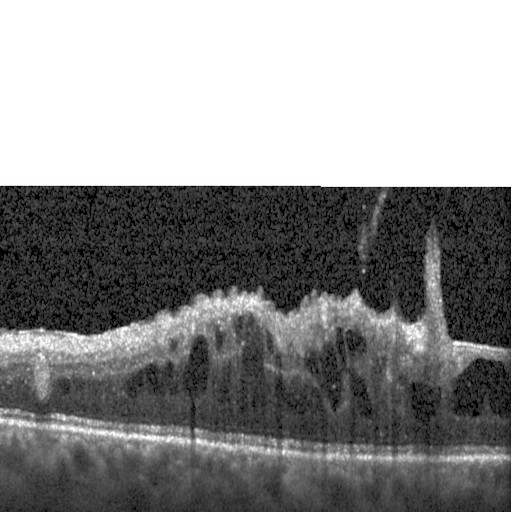
Finding: diabetic macular edema (DME).